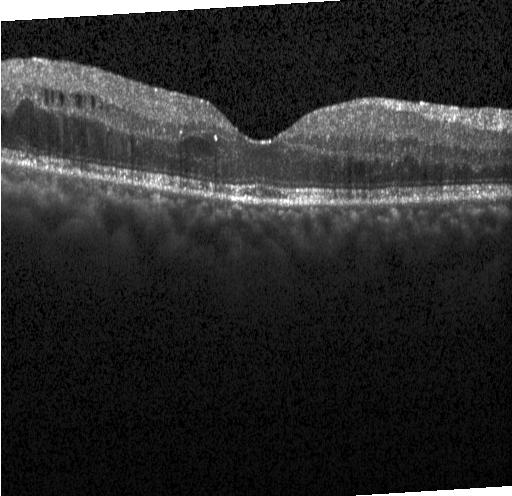 Diagnosis: diabetic macular edema (DME).